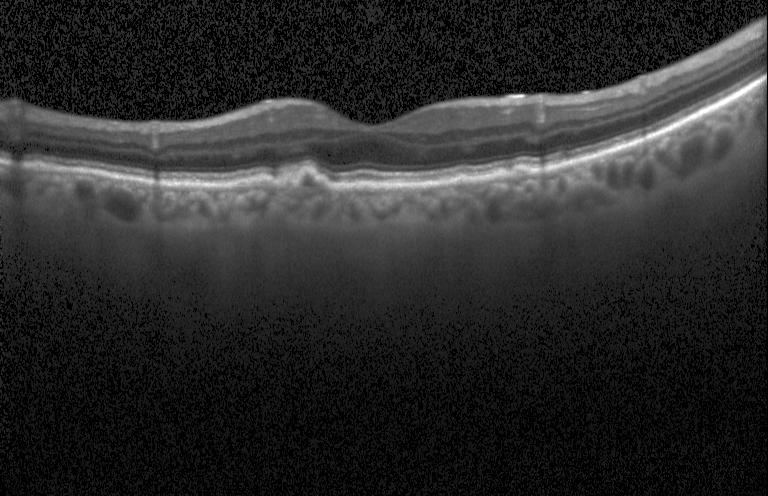

Diagnosis: sub-RPE drusenoid deposits.